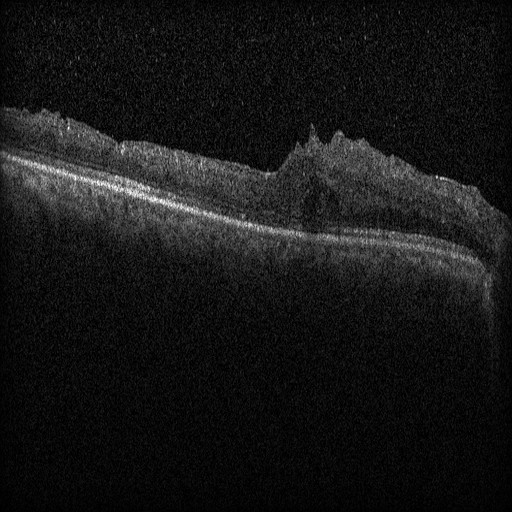

Assessment: DME.